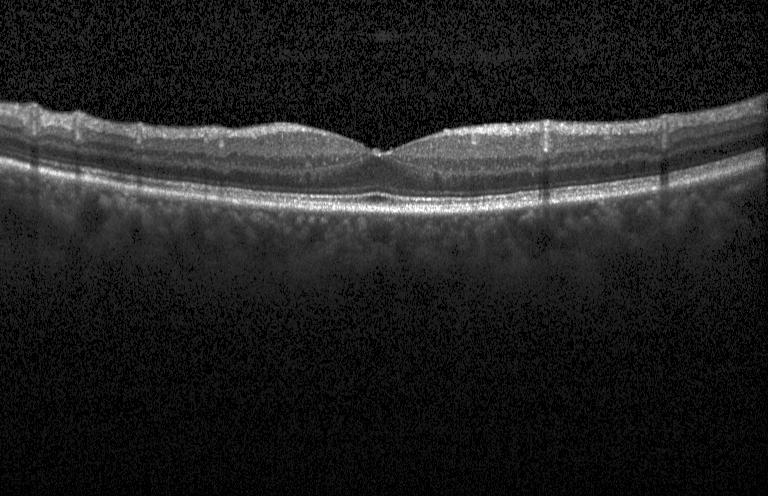

Optical coherence tomography B-scan; spectral-domain optical coherence tomography. This B-scan demonstrates no evidence of CNV, DME, or drusen.